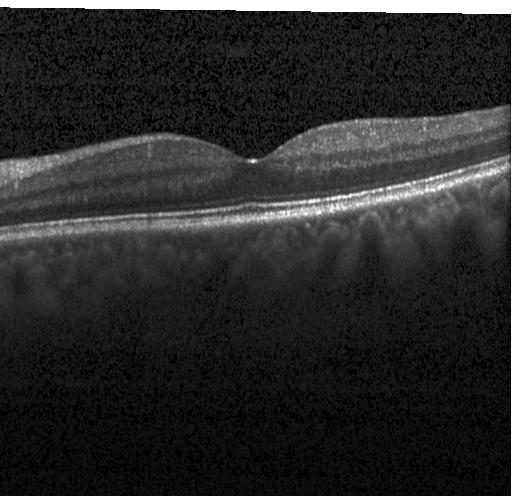

Finding: no CNV, DME, or drusen.